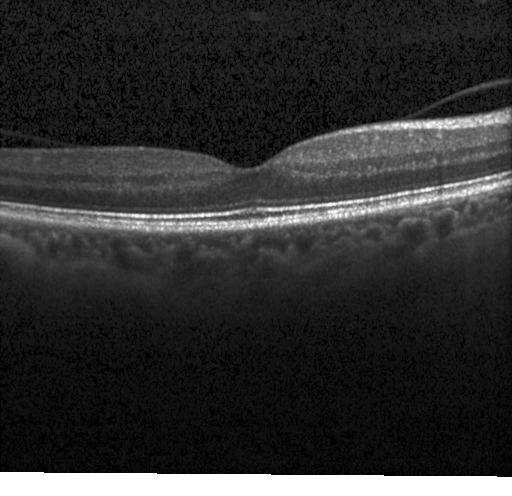
OCT B-scan.
Dx: no CNV, DME, or drusen.